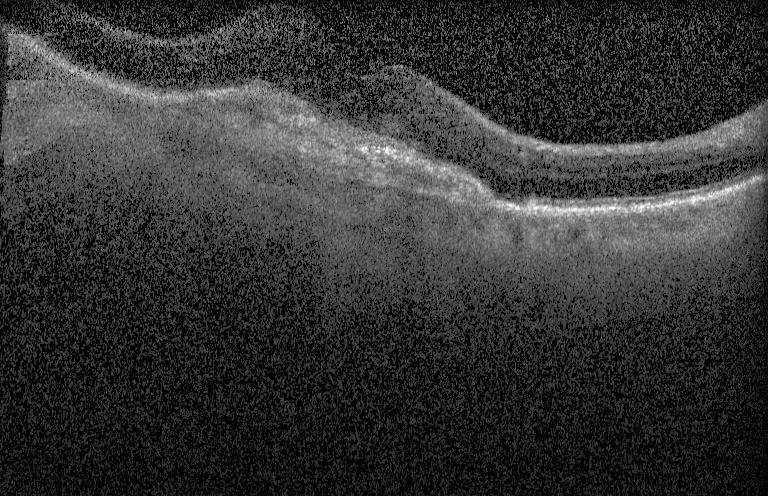 Optical coherence tomography B-scan, horizontal scan through the fovea, Heidelberg Spectralis OCT system
Assessment: CNV.